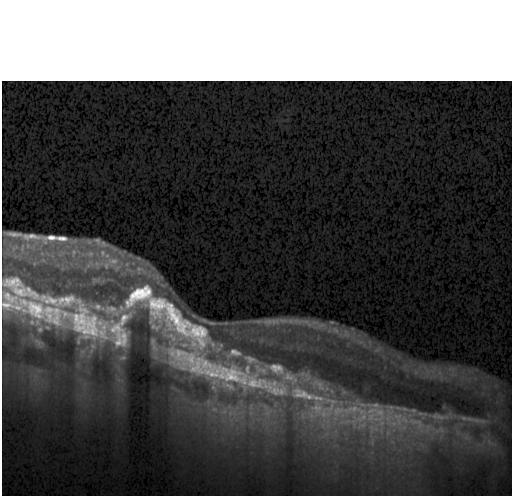 Retinal OCT cross-section showing a choroidal neovascular membrane.